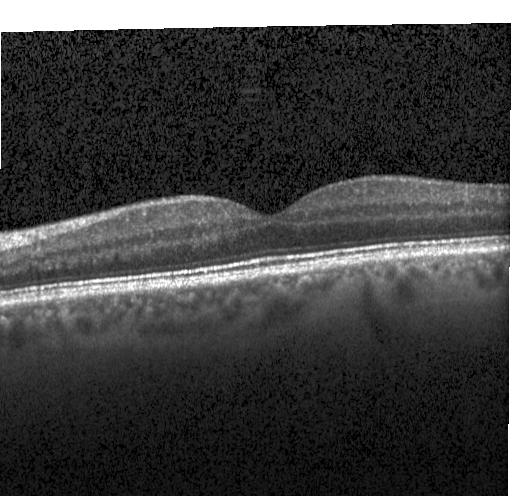 Horizontal scan through the fovea. Retinal OCT B-scan. Heidelberg Spectralis. SD-OCT — No CNV, DME, or drusen.